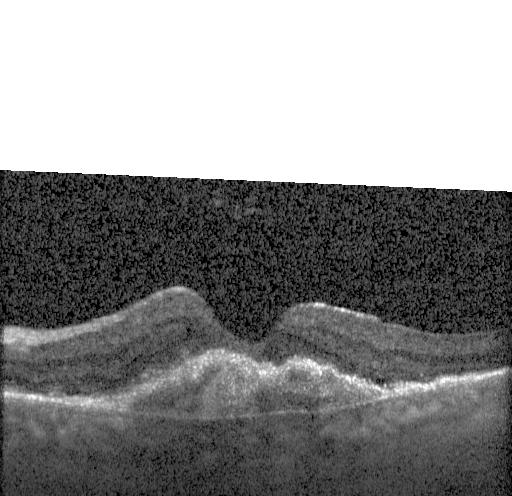
OCT scan showing a choroidal neovascular membrane.